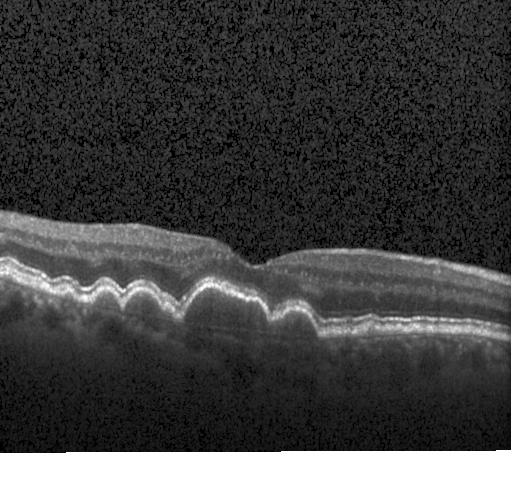
SD-OCT; acquired on a Heidelberg Spectralis; OCT B-scan; fovea-centered
Multiple drusen.